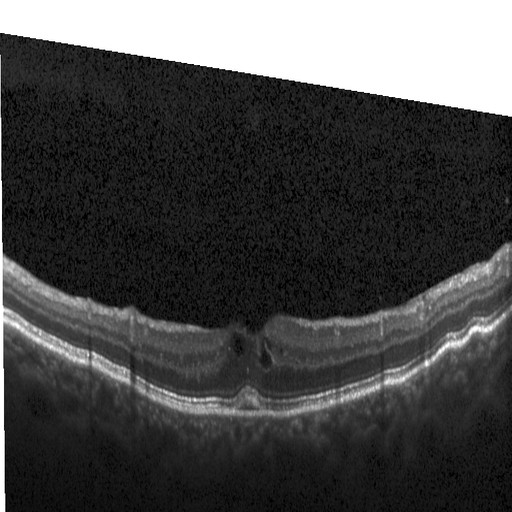
OCT finding: diabetic macular edema (DME).